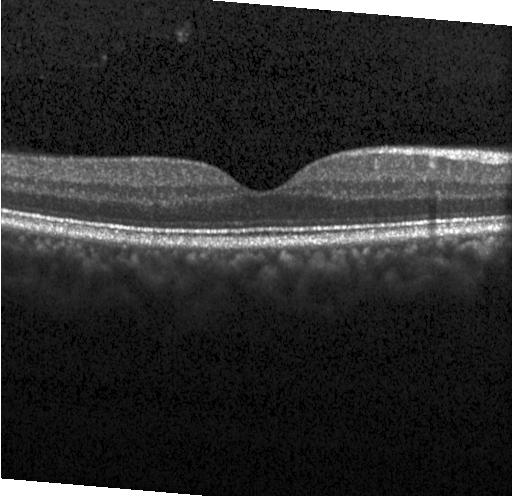 Macular scan, instrument: Heidelberg Spectralis, optical coherence tomography B-scan — Finding: neither choroidal neovascularization, diabetic macular edema, nor drusen.